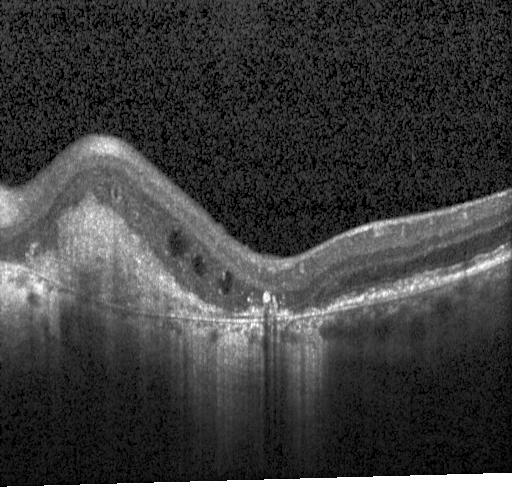
Diagnosis: CNV.